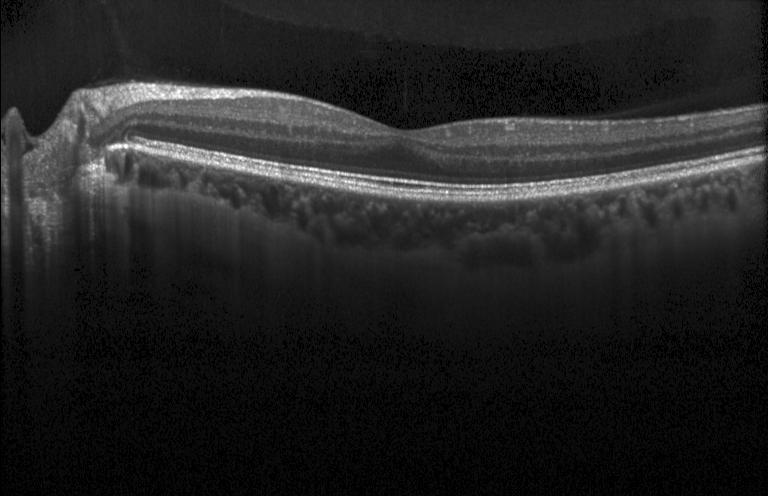
Diagnosis: no evidence of CNV, DME, or drusen.